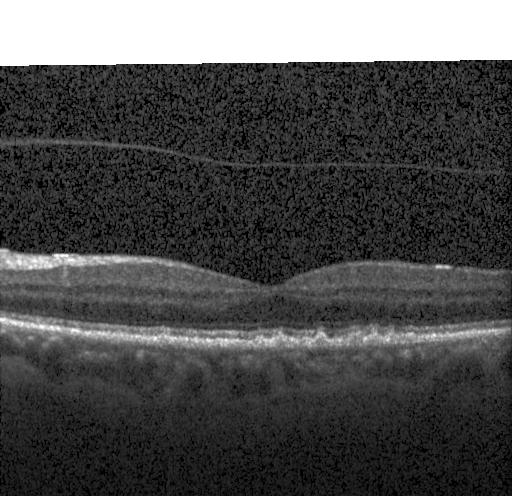

OCT B-scan; centered on the fovea; Heidelberg Spectralis; SD-OCT.
Diagnosis: sub-RPE drusenoid deposits.